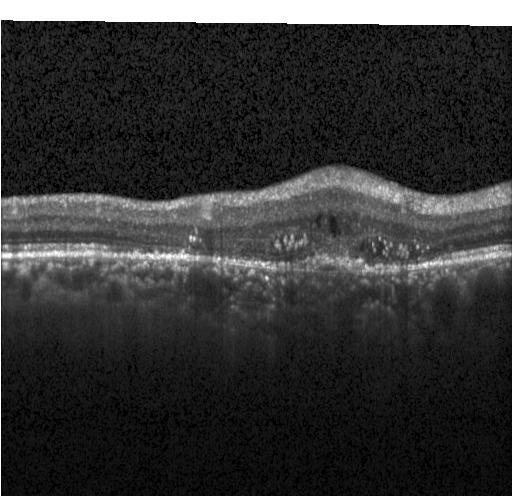

Impression: a choroidal neovascular membrane.